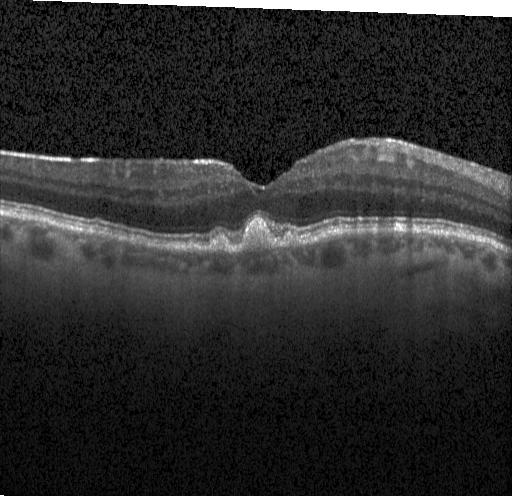

Optical coherence tomography B-scan; Heidelberg Spectralis; through the macula
Assessment: sub-RPE drusenoid deposits.